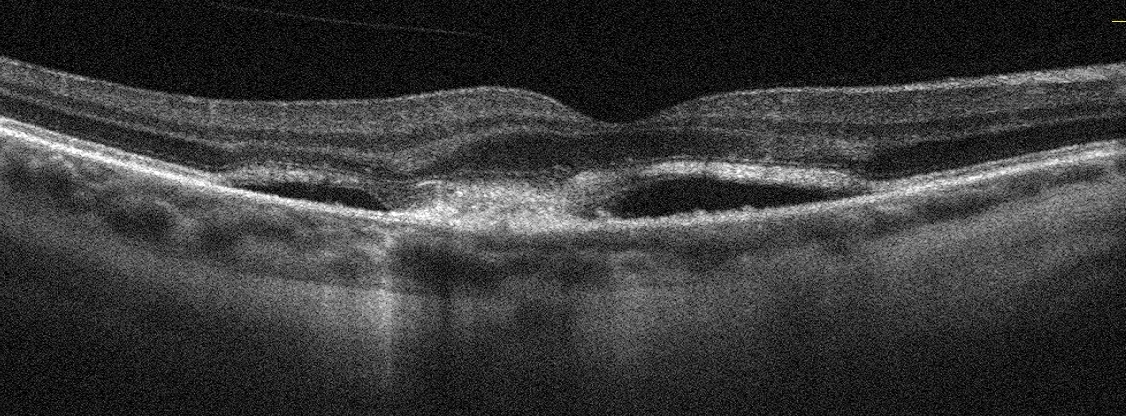

Macular scan, retinal OCT cross-section.
This B-scan demonstrates AMD.